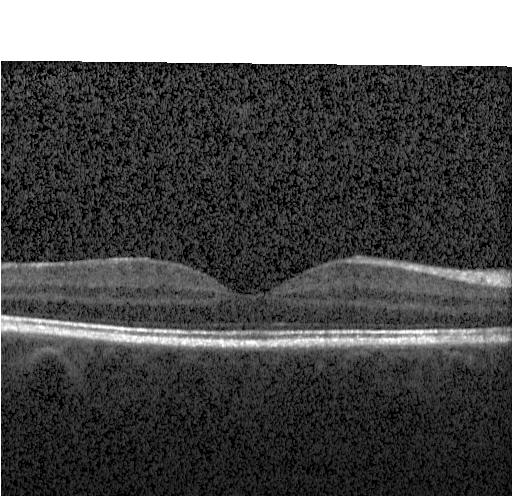
Macular OCT demonstrating no choroidal neovascularization, no diabetic macular edema, and no drusen.